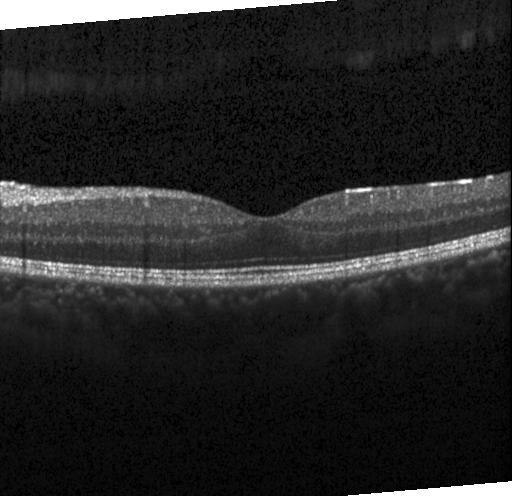
Assessment: no choroidal neovascularization, diabetic macular edema, or drusen.